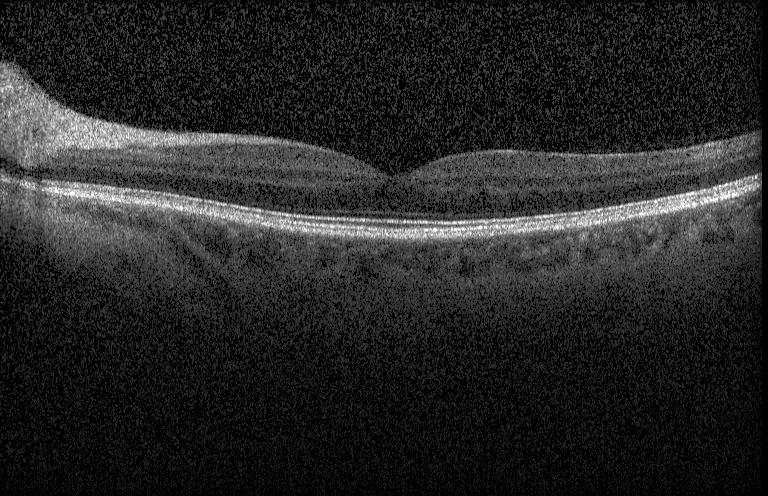

Heidelberg Spectralis. Horizontal scan through the fovea. Spectral-domain optical coherence tomography. Retinal OCT cross-section
Diagnosis: no evidence of choroidal neovascularization, diabetic macular edema, or drusen.